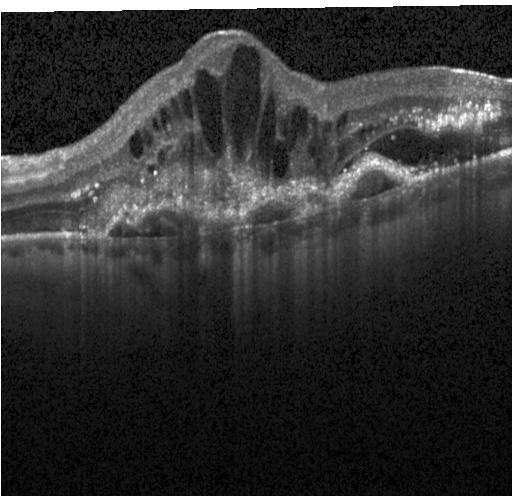 Dx: choroidal neovascularization (CNV).